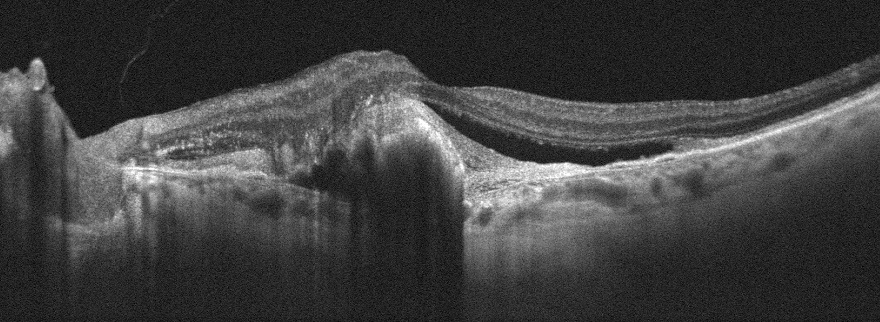 OCT finding: age-related macular degeneration (AMD).